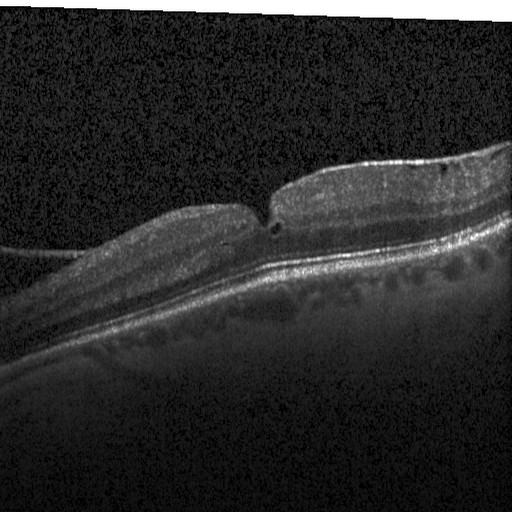

Instrument: Heidelberg Spectralis, OCT line scan, fovea-centered, SD-OCT
OCT finding: diabetic macular edema.